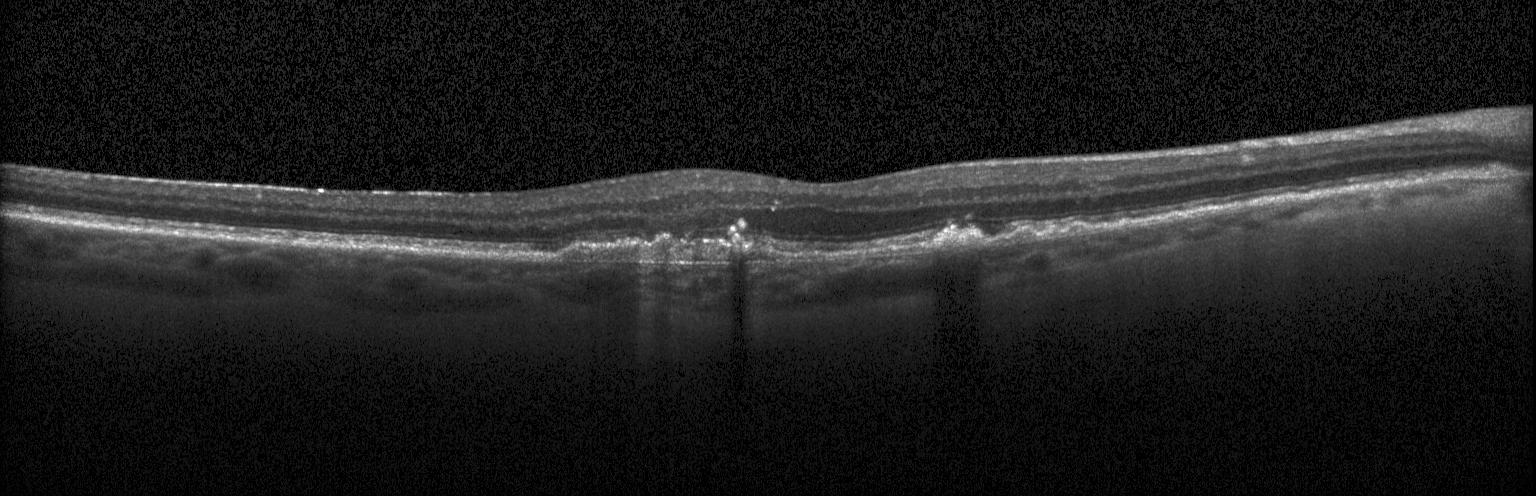
Diagnosis: a choroidal neovascular membrane.